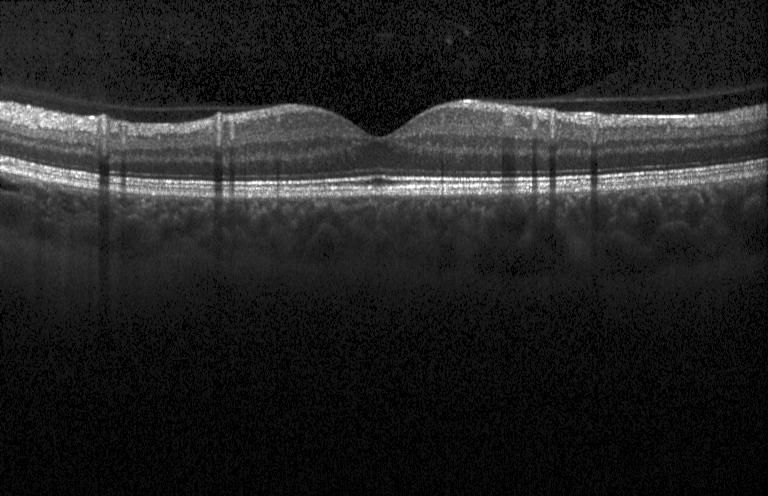
Optical coherence tomography scan · instrument: Heidelberg Spectralis. Diagnosis: no choroidal neovascularization, no diabetic macular edema, and no drusen.